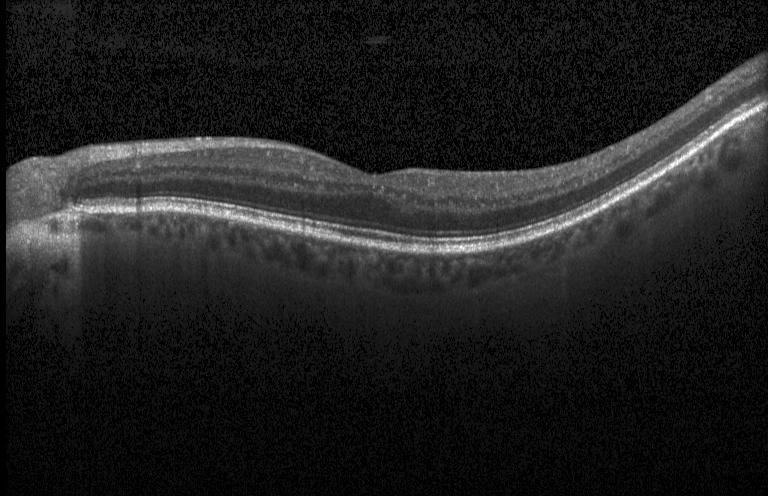
Acquired on a Heidelberg Spectralis; retinal OCT B-scan; macular scan
This B-scan demonstrates neither choroidal neovascularization, diabetic macular edema, nor drusen.